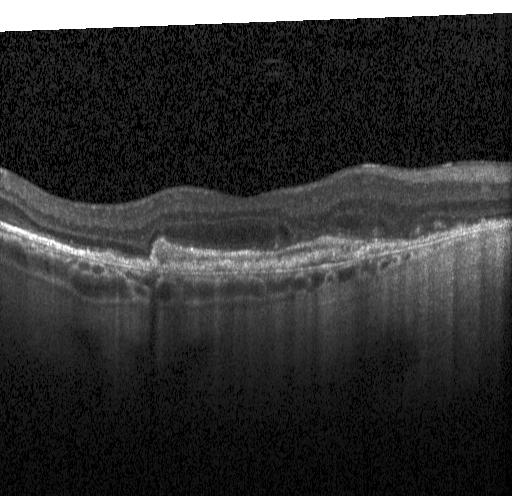

Retinal OCT cross-section; SD-OCT.
Macular OCT: a choroidal neovascular membrane.